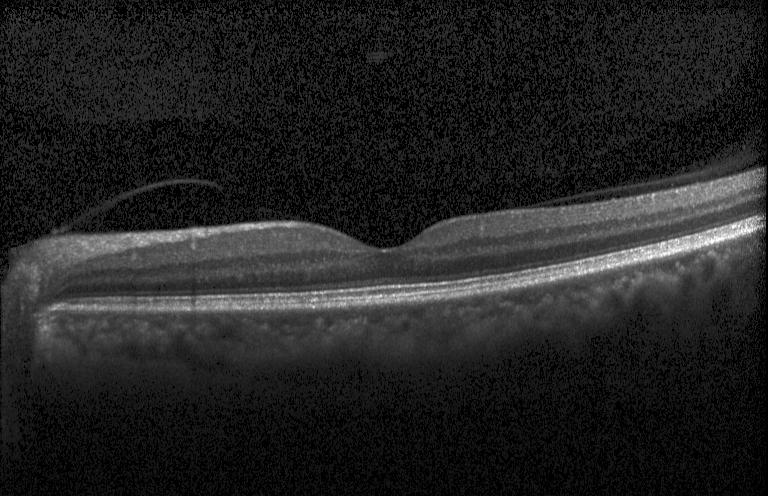

OCT B-scan showing no choroidal neovascularization, diabetic macular edema, or drusen.